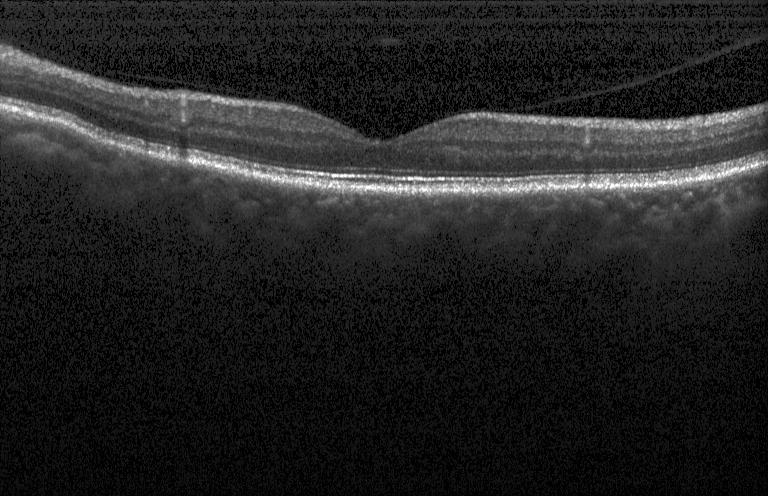 Assessment: no evidence of CNV, DME, or drusen.